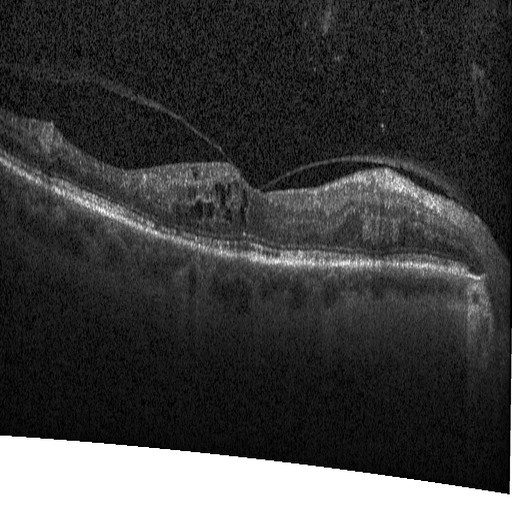

Heidelberg Spectralis OCT system, optical coherence tomography scan, centered on the fovea, spectral-domain optical coherence tomography — The scan shows diabetic macular edema.